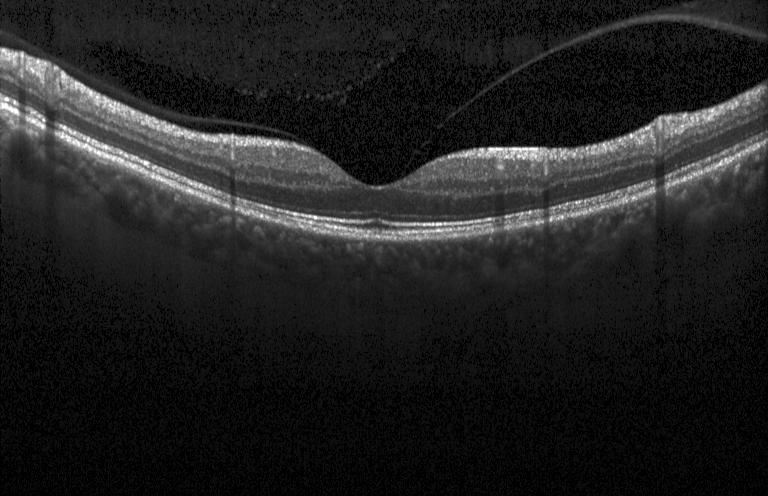 OCT scan showing no choroidal neovascularization, diabetic macular edema, or drusen.